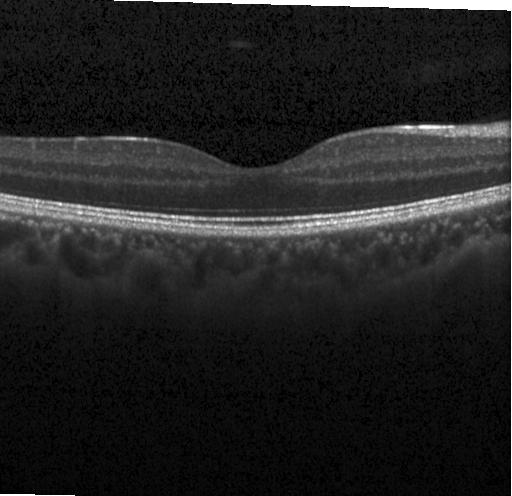

Retinal OCT cross-section showing neither choroidal neovascularization, diabetic macular edema, nor drusen.